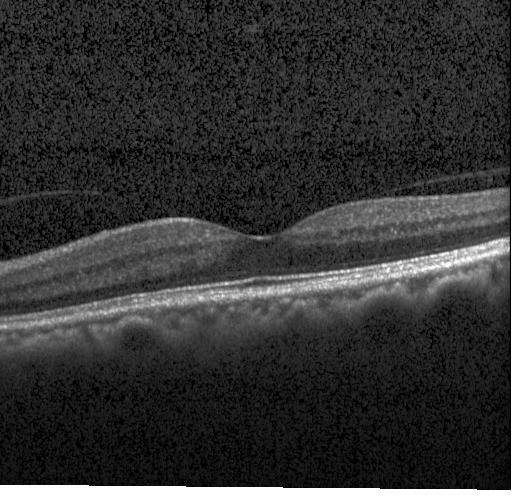 Finding: neither choroidal neovascularization, diabetic macular edema, nor drusen.